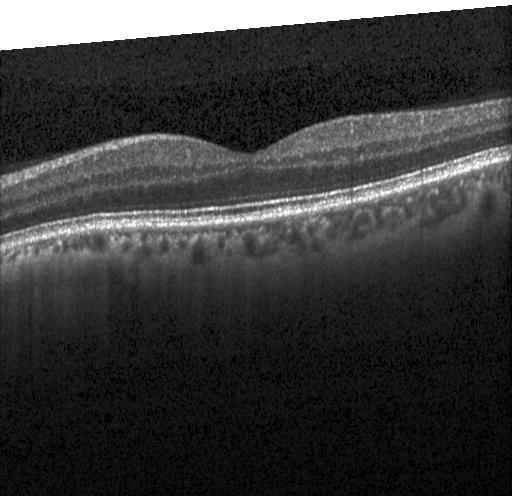 OCT B-scan.
Diagnosis: no CNV, no DME, and no drusen.